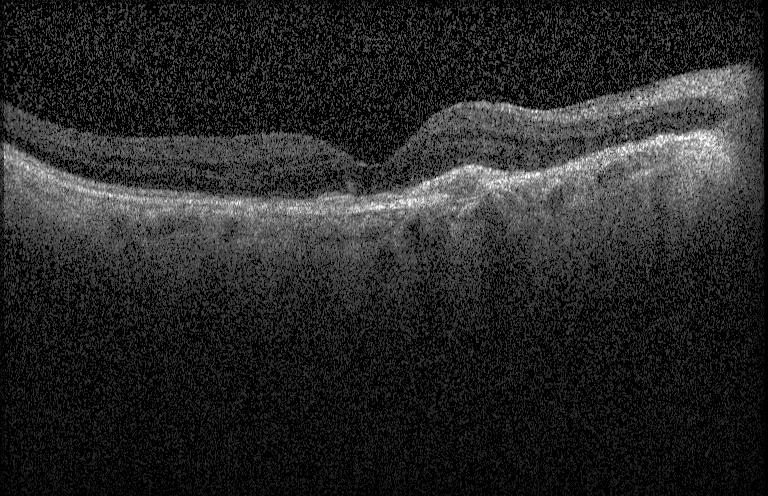

SD-OCT · optical coherence tomography scan. This B-scan demonstrates CNV.